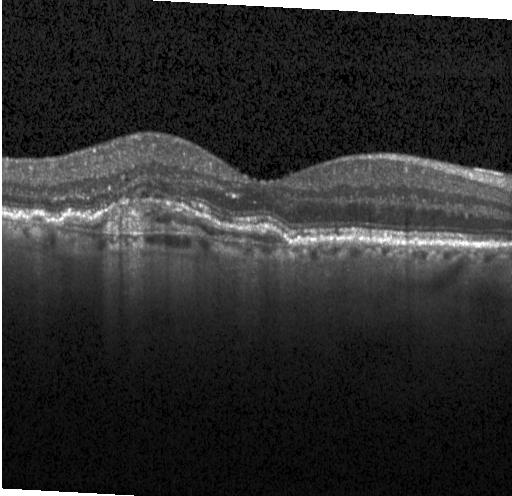
Heidelberg Spectralis OCT system; OCT B-scan; macular scan — This B-scan demonstrates a choroidal neovascular membrane.